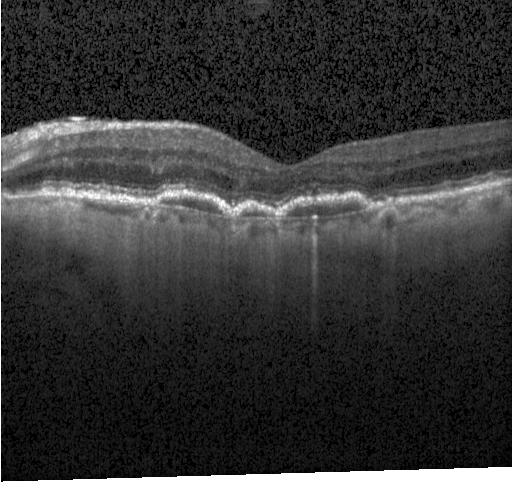
Centered on the fovea. Optical coherence tomography B-scan.
Diagnosis: a choroidal neovascular membrane.